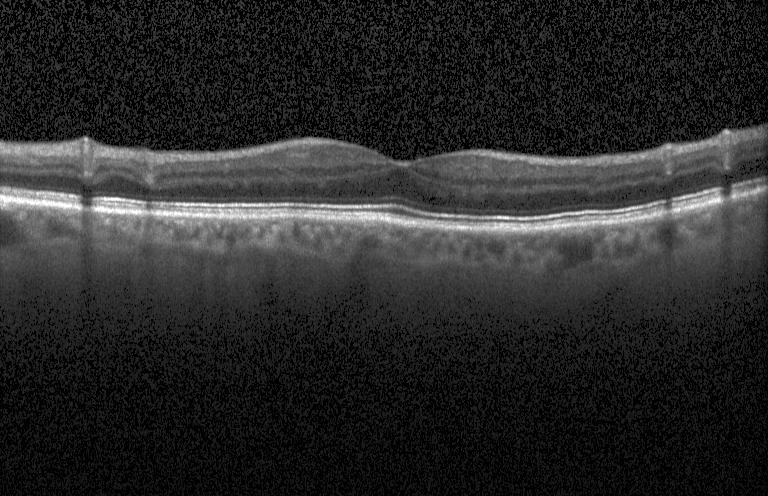
Finding: no choroidal neovascularization, diabetic macular edema, or drusen.